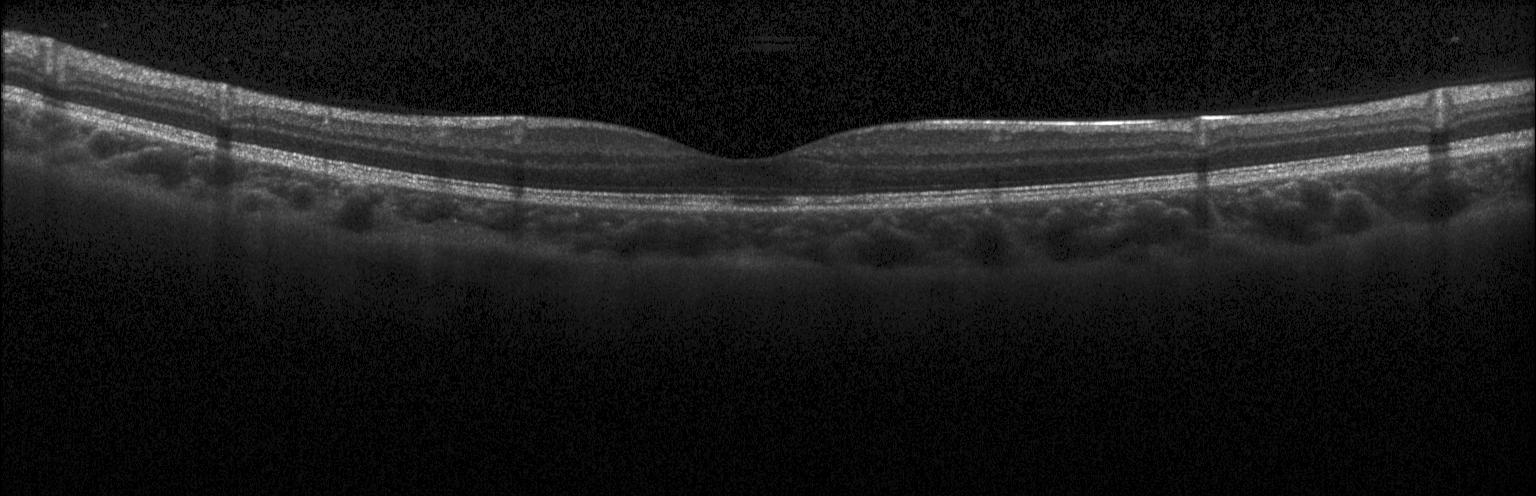

OCT line scan; macular scan — The scan shows no evidence of choroidal neovascularization, diabetic macular edema, or drusen.